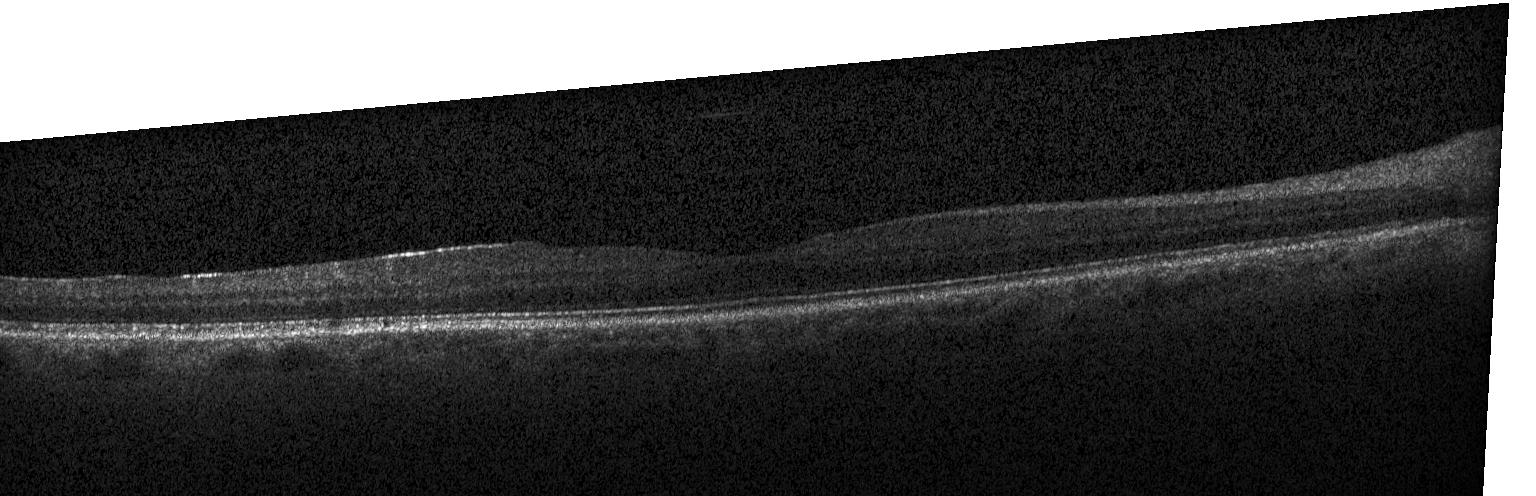
Centered on the fovea, spectral-domain optical coherence tomography, instrument: Heidelberg Spectralis, optical coherence tomography B-scan. Finding: no choroidal neovascularization, diabetic macular edema, or drusen.